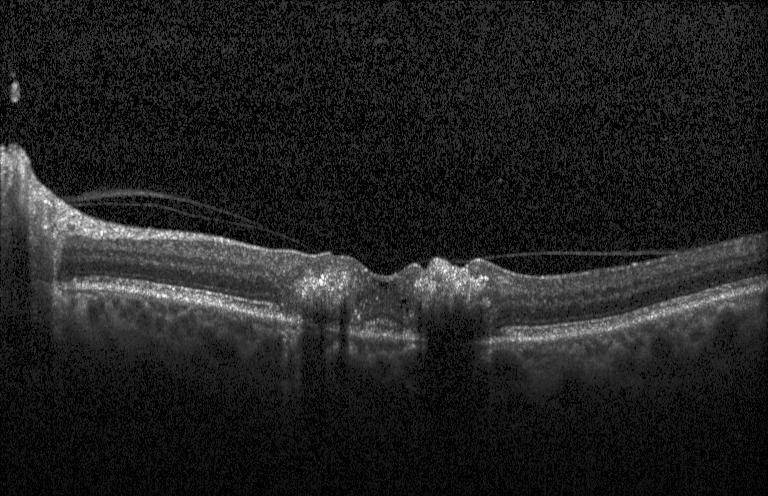 Spectral-domain OCT B-scan: CNV.